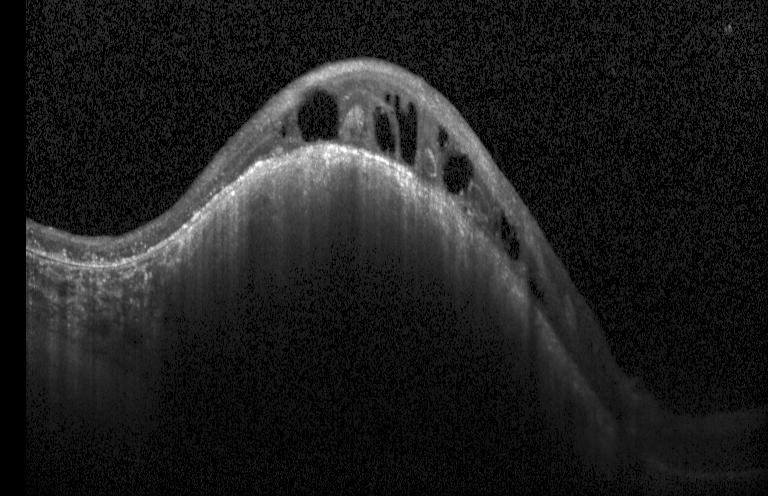
Retinal OCT B-scan.
Impression: diabetic macular edema (DME).